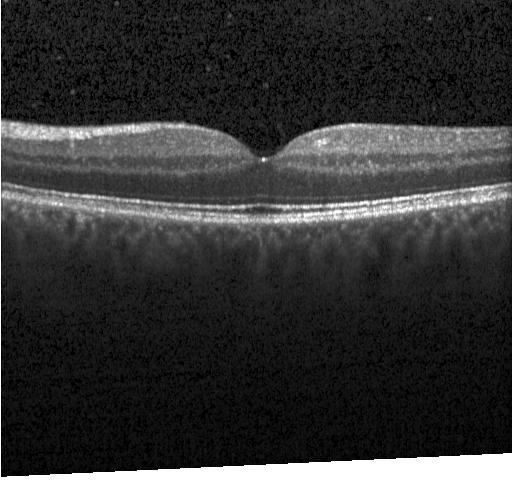

Spectral-domain OCT, OCT B-scan. Diagnosis: no choroidal neovascularization, no diabetic macular edema, and no drusen.